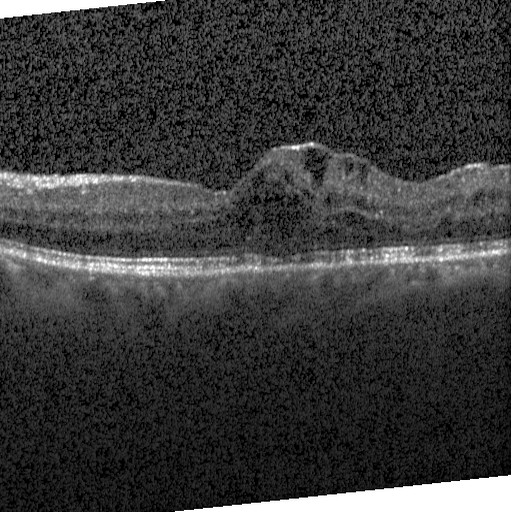

SD-OCT · fovea-centered · retinal OCT cross-section — Assessment: diabetic macular edema.